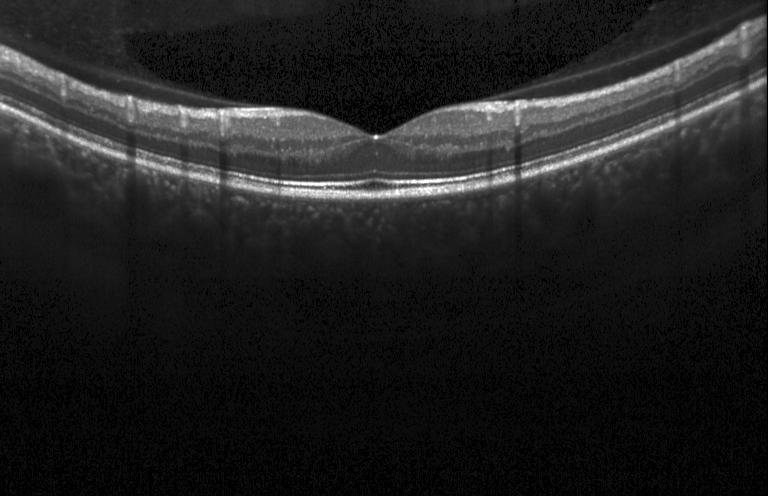 Centered on the fovea; optical coherence tomography B-scan. This B-scan demonstrates no choroidal neovascularization, no diabetic macular edema, and no drusen.